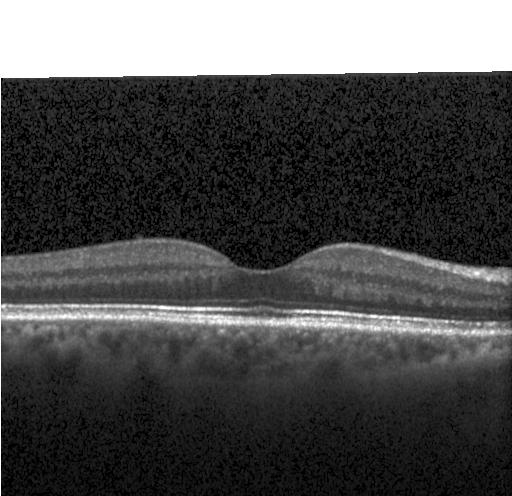 Spectral-domain OCT · retinal OCT B-scan · centered on the fovea — No choroidal neovascularization, no diabetic macular edema, and no drusen.